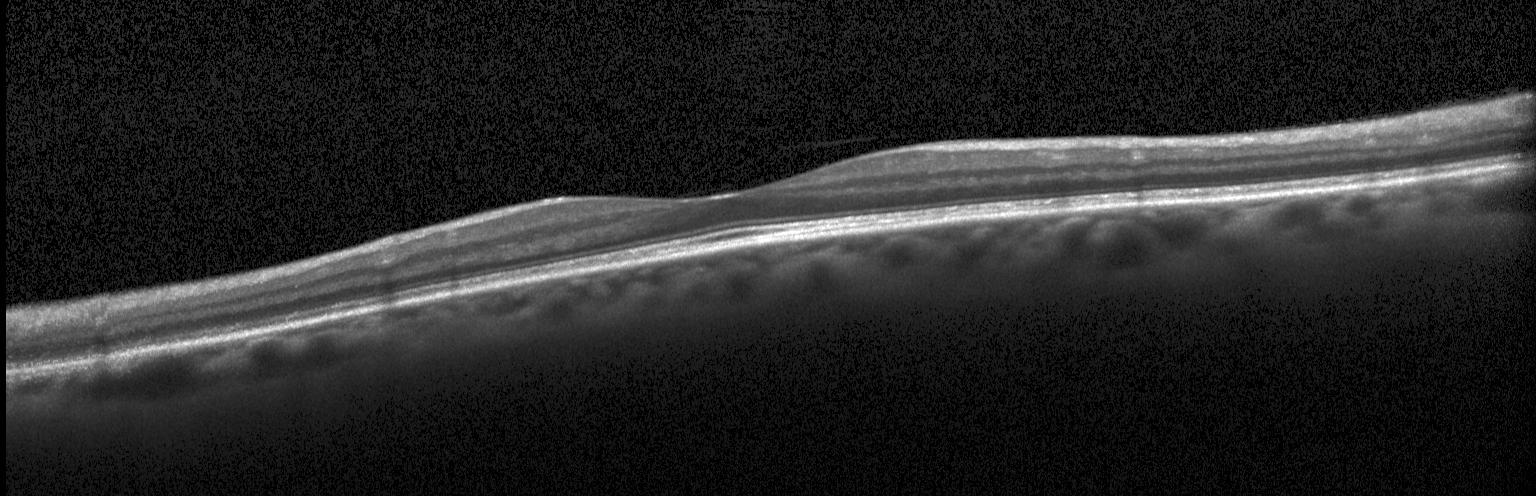

Macular OCT demonstrating neither choroidal neovascularization, diabetic macular edema, nor drusen.